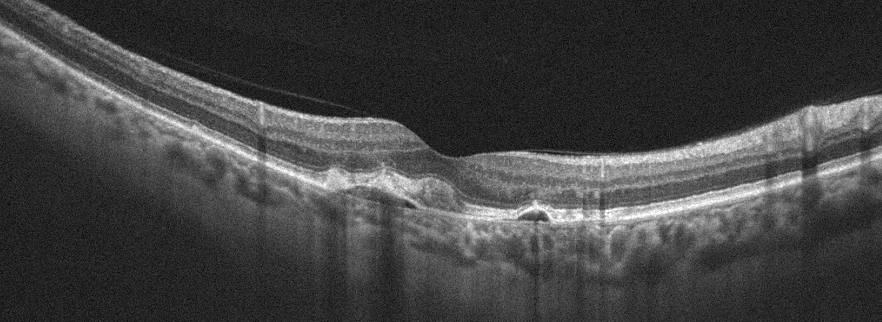 Retinal OCT B-scan; oculus dexter.
This B-scan demonstrates AMD.